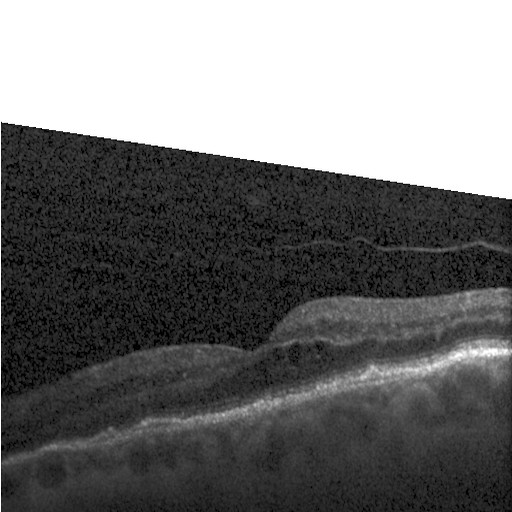 Macular scan; OCT B-scan.
This B-scan demonstrates diabetic macular edema (DME).